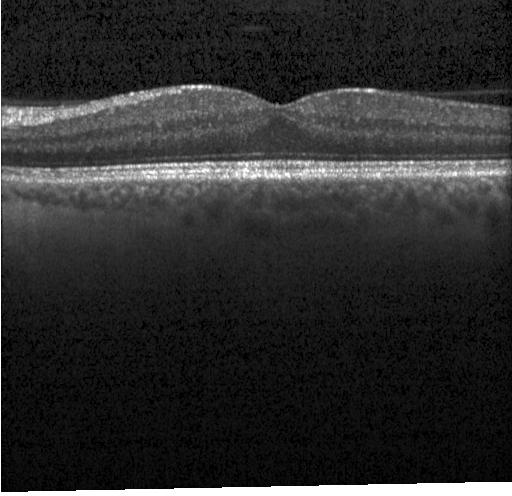
Retinal OCT B-scan; through the macula; spectral-domain optical coherence tomography. Impression: no CNV, DME, or drusen.